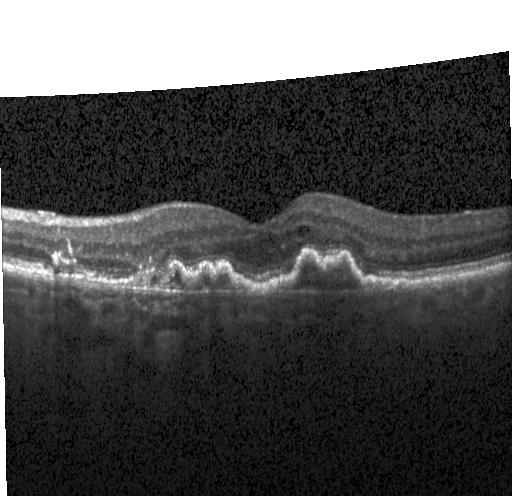
Retinal OCT cross-section. SD-OCT — Choroidal neovascularization (CNV).